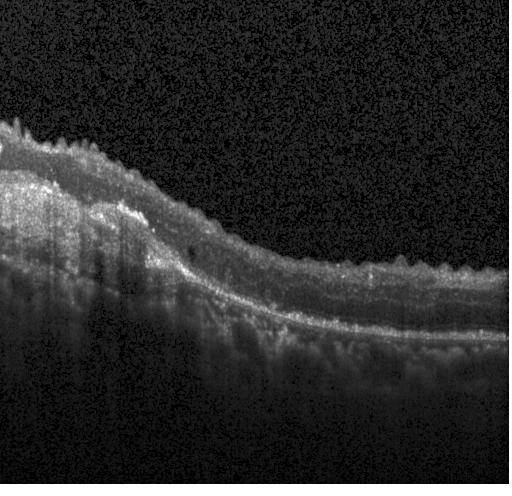 SD-OCT. Heidelberg Spectralis. Through the macula. OCT line scan. Finding: CNV.